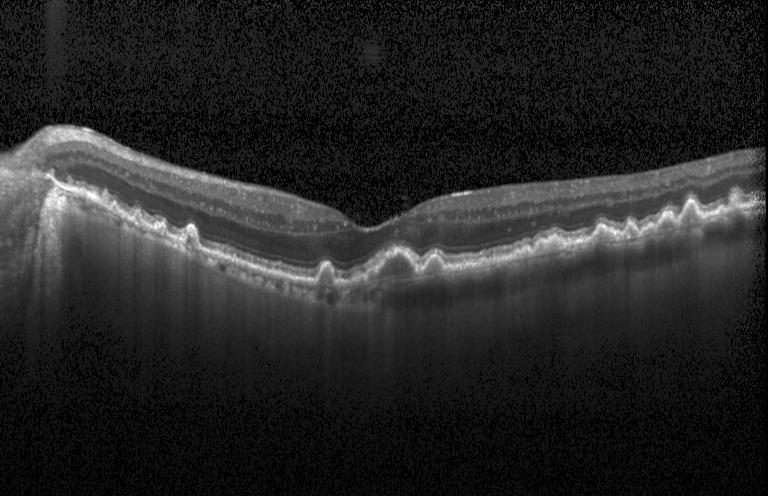

Optical coherence tomography B-scan. Heidelberg Spectralis OCT system. Centered on the fovea. OCT finding: multiple drusen.